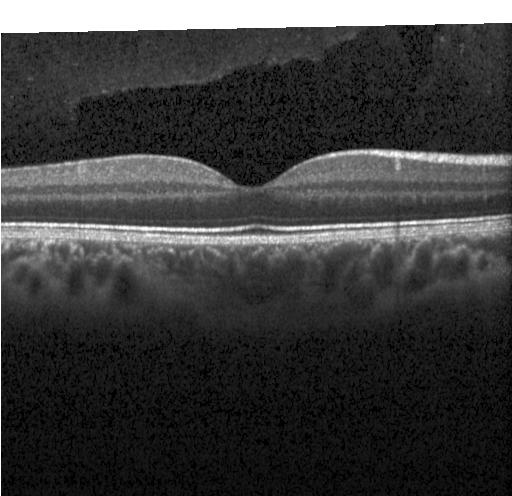
Impression: no choroidal neovascularization, no diabetic macular edema, and no drusen.